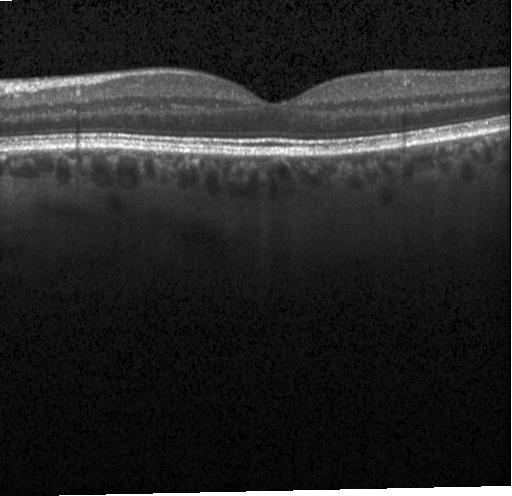
Centered on the fovea, optical coherence tomography scan. Macular OCT: no evidence of CNV, DME, or drusen.